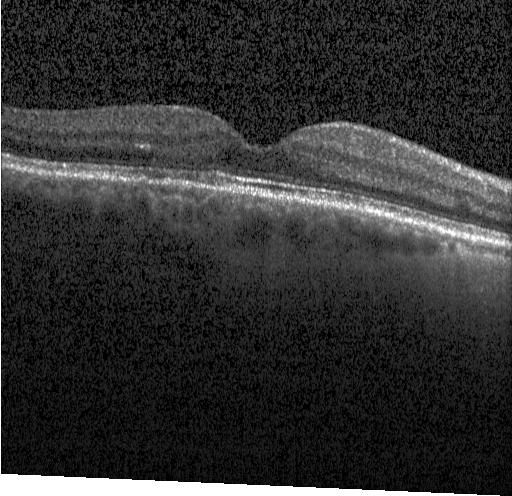

Spectral-domain optical coherence tomography. Horizontal scan through the fovea. Optical coherence tomography scan. Heidelberg Spectralis OCT system — Assessment: no choroidal neovascularization, no diabetic macular edema, and no drusen.